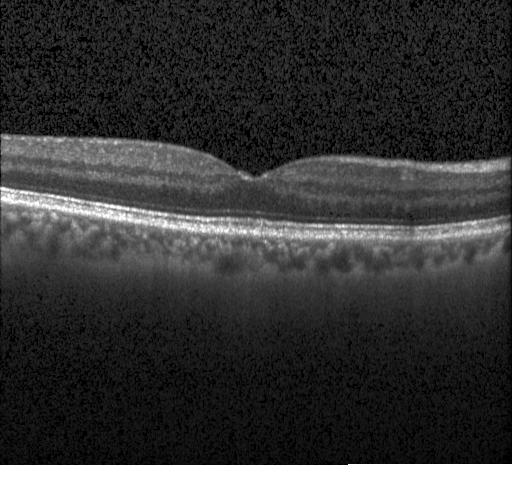
Macular OCT: no CNV, DME, or drusen.